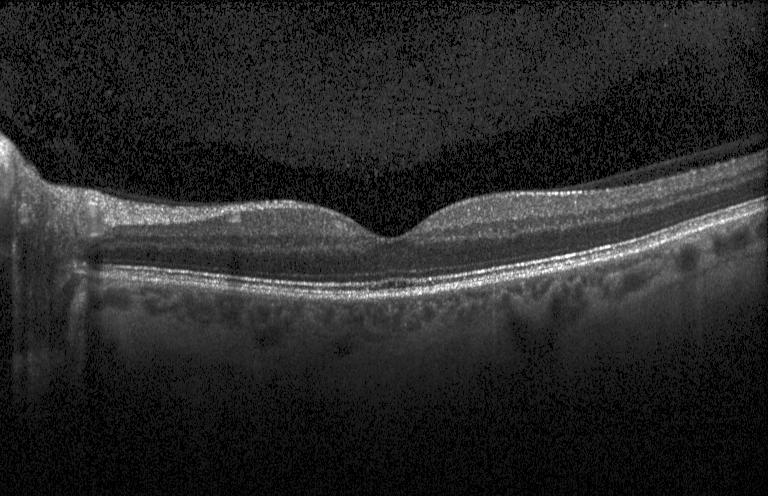

OCT line scan, acquired on a Heidelberg Spectralis.
Diagnosis: no choroidal neovascularization, no diabetic macular edema, and no drusen.